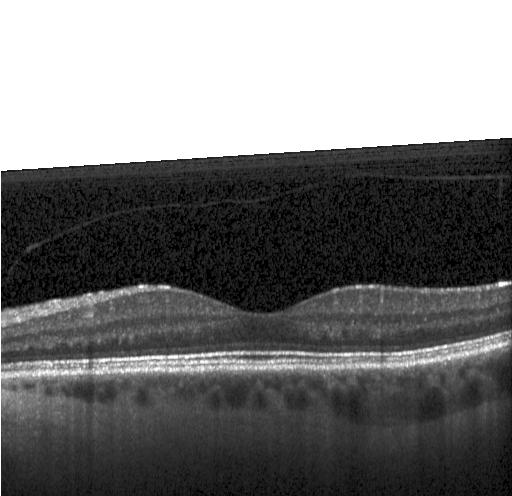 Impression: neither choroidal neovascularization, diabetic macular edema, nor drusen.